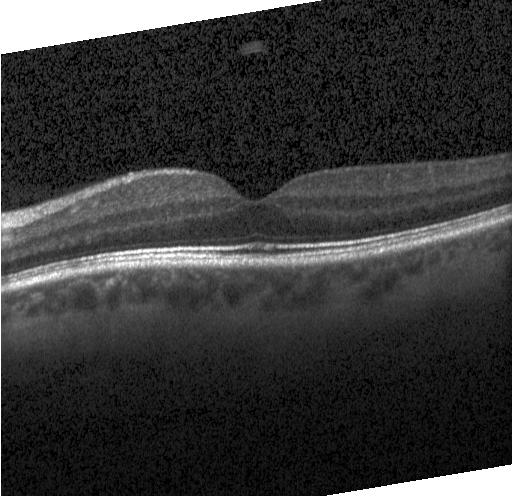

Heidelberg Spectralis, fovea-centered, retinal OCT B-scan, SD-OCT
Finding: no evidence of CNV, DME, or drusen.